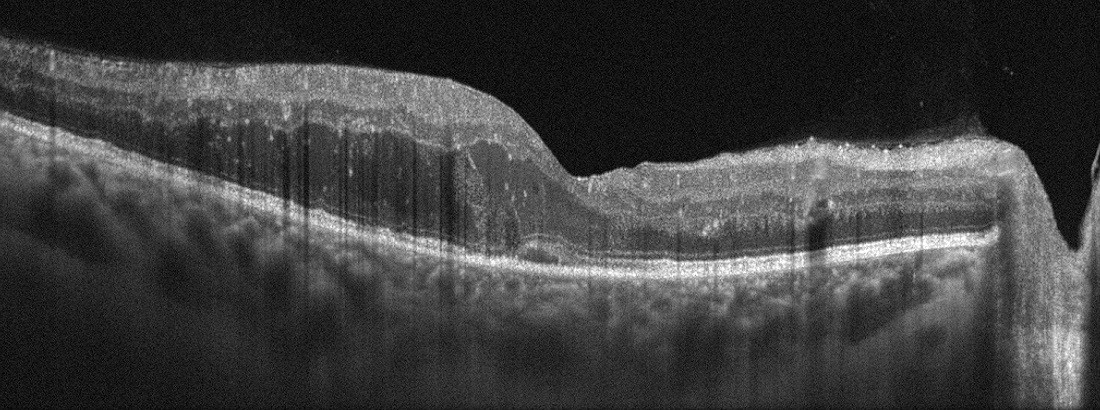
OCT B-scan showing diabetic macular edema.